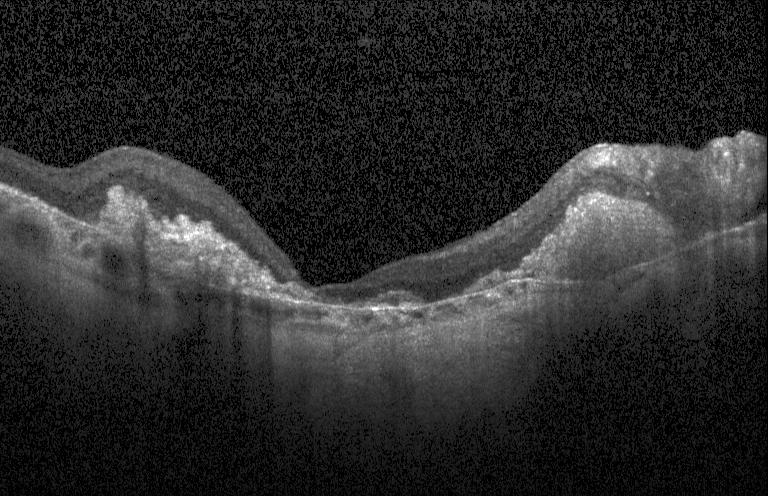
Impression: choroidal neovascularization (CNV).